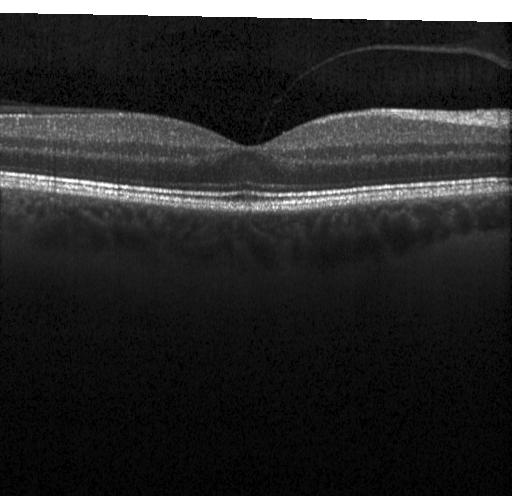 This B-scan demonstrates no evidence of choroidal neovascularization, diabetic macular edema, or drusen.